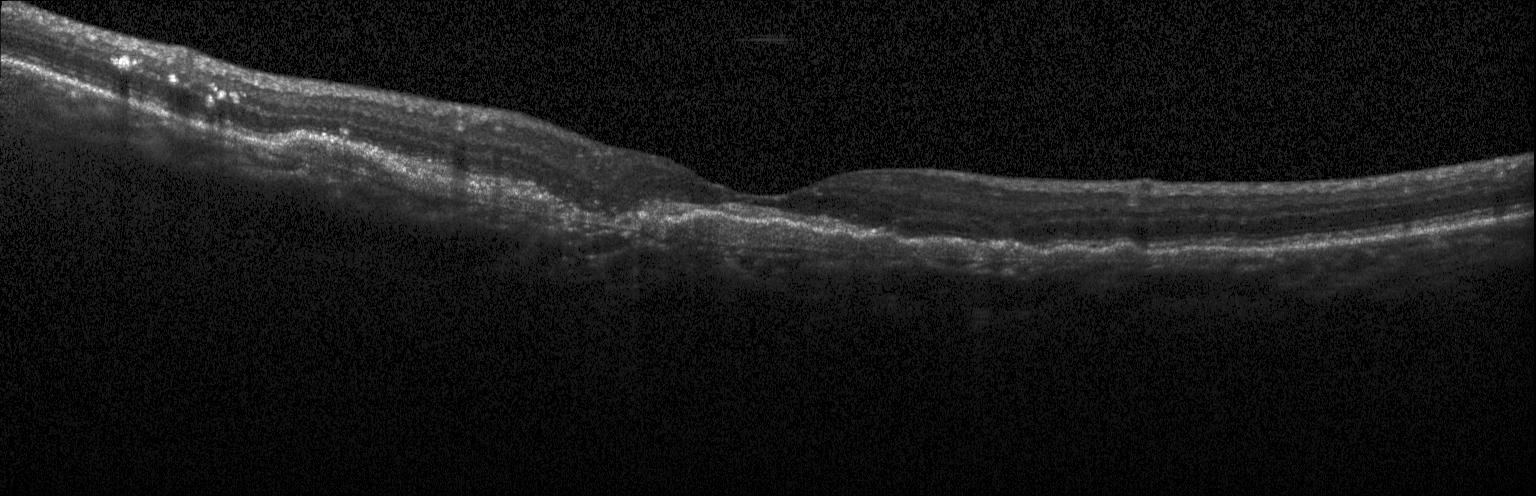
OCT line scan
Choroidal neovascularization (CNV).